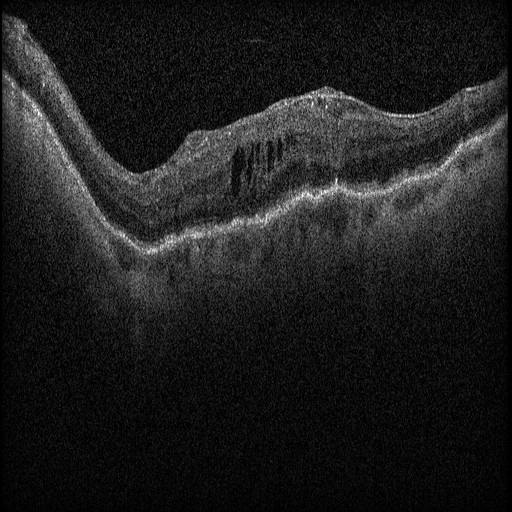
Optical coherence tomography scan.
Diabetic macular edema.